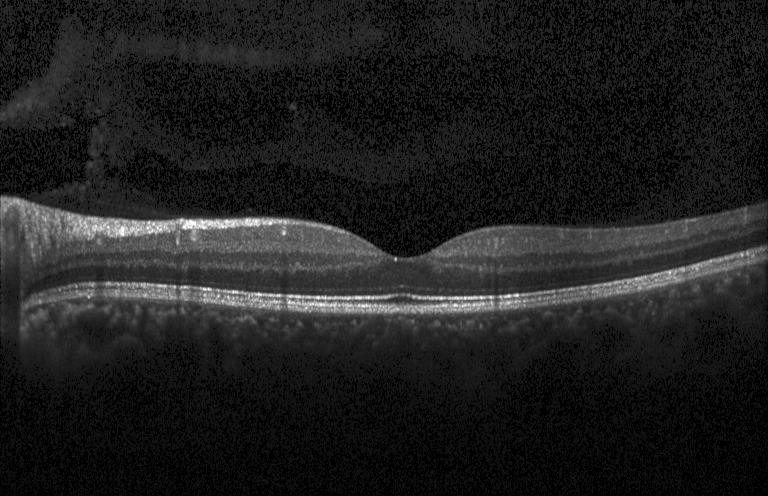 OCT B-scan showing no CNV, no DME, and no drusen.